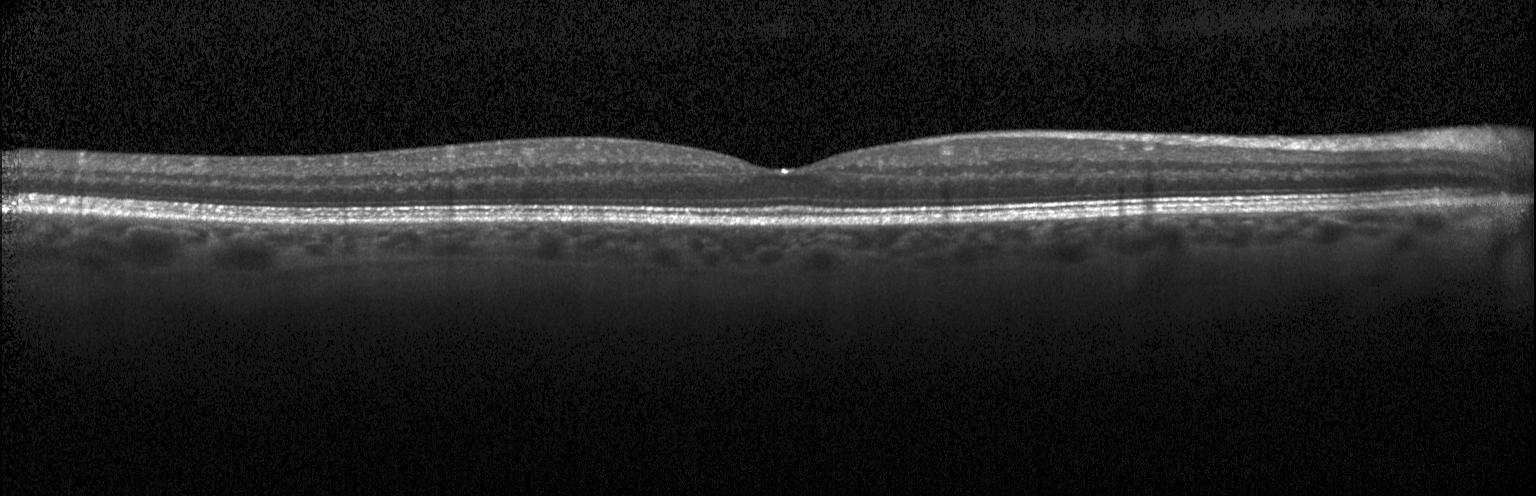
Diagnosis: no choroidal neovascularization, diabetic macular edema, or drusen.